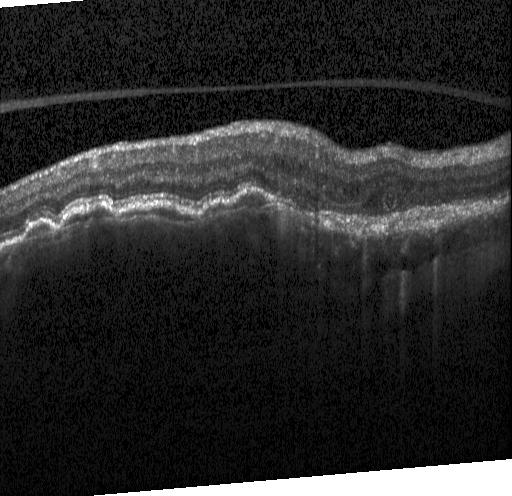
Diagnosis: a choroidal neovascular membrane.